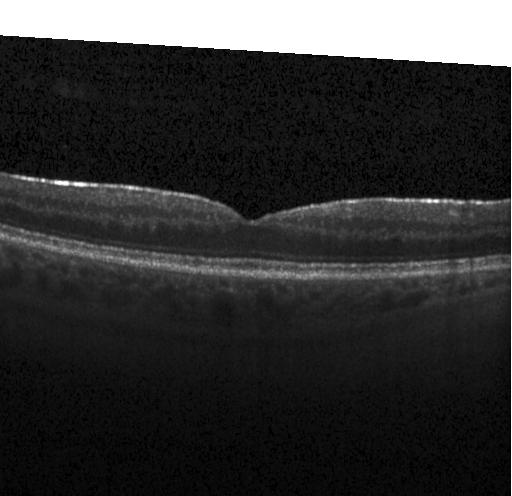 Macular OCT: neither choroidal neovascularization, diabetic macular edema, nor drusen.